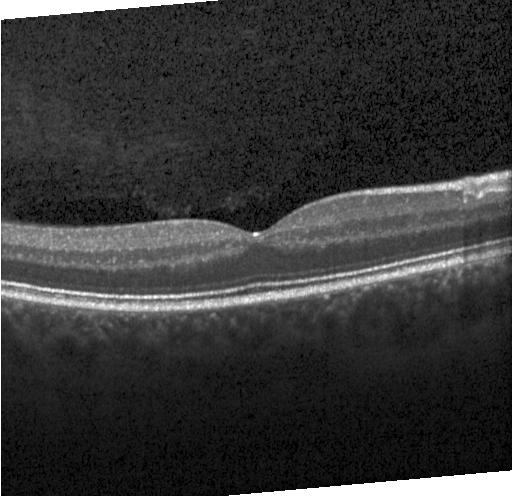 Spectral-domain optical coherence tomography; Heidelberg Spectralis; OCT line scan. Dx: no choroidal neovascularization, no diabetic macular edema, and no drusen.